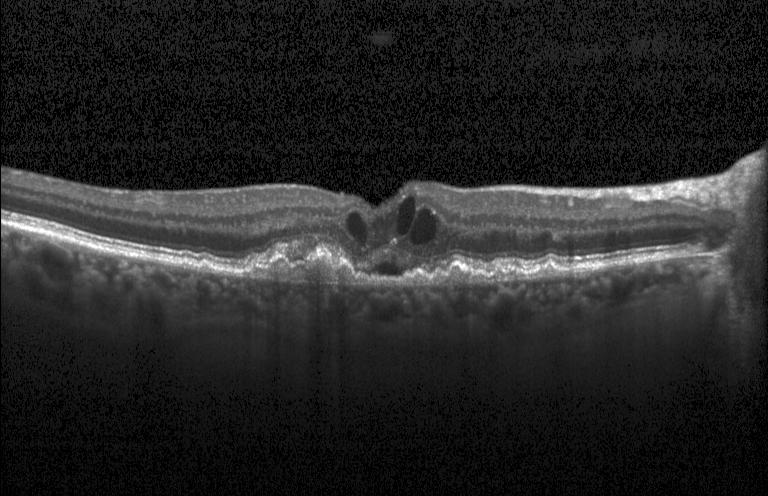
Spectral-domain OCT · OCT line scan. Impression: choroidal neovascularization.